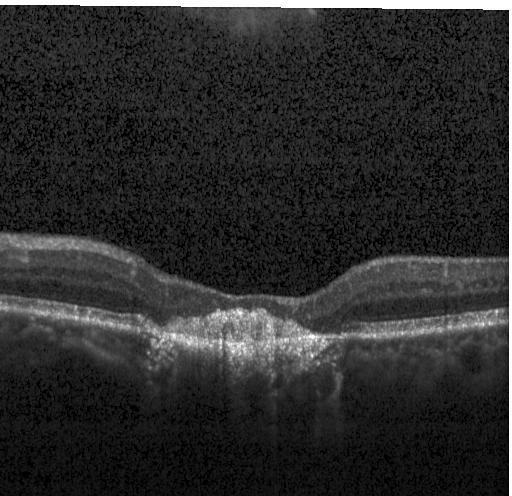 OCT scan showing CNV.